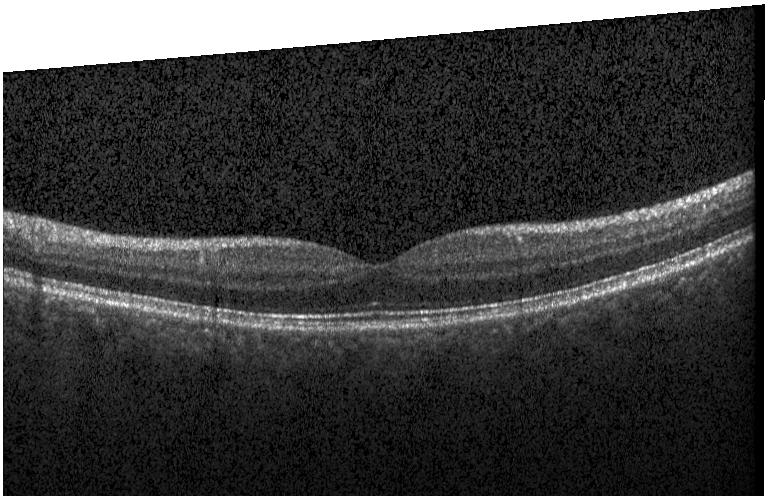

Impression: no CNV, DME, or drusen.